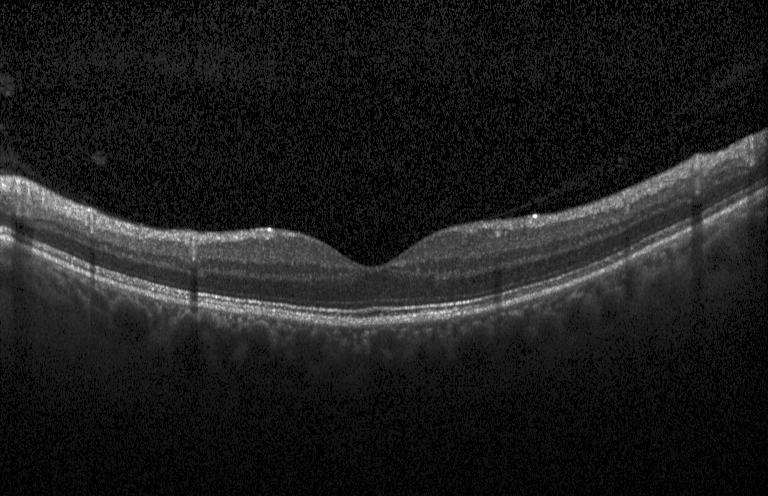 Heidelberg Spectralis, OCT B-scan, spectral-domain OCT, fovea-centered.
Finding: neither choroidal neovascularization, diabetic macular edema, nor drusen.